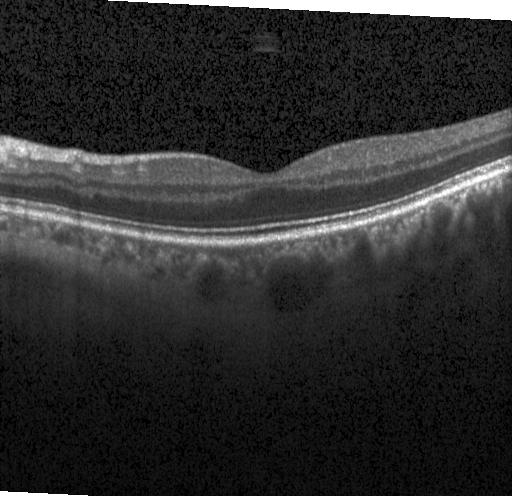 Optical coherence tomography scan — Assessment: no choroidal neovascularization, diabetic macular edema, or drusen.